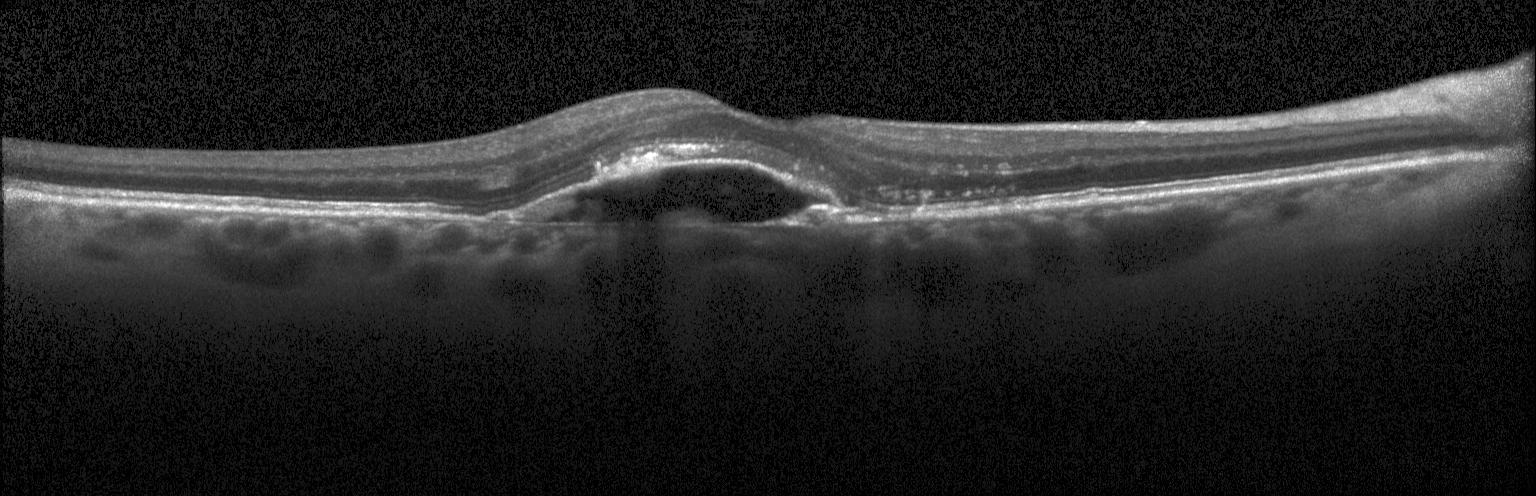 Macular OCT demonstrating choroidal neovascularization (CNV).